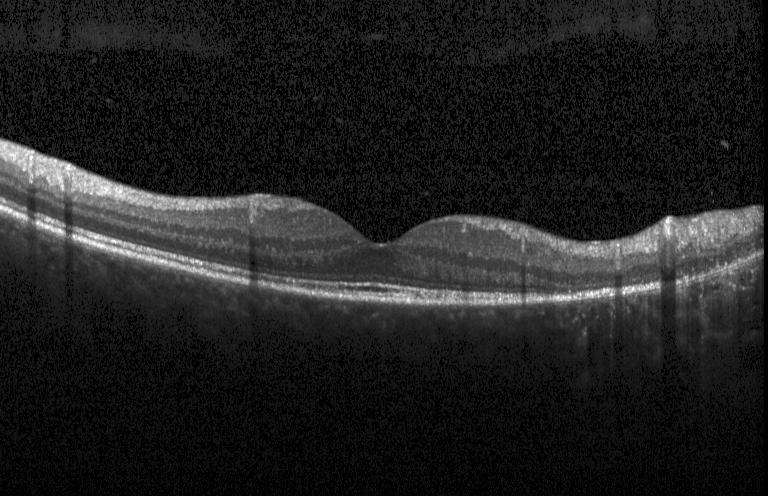 Through the macula; SD-OCT; optical coherence tomography scan; acquired on a Heidelberg Spectralis — Finding: no evidence of choroidal neovascularization, diabetic macular edema, or drusen.